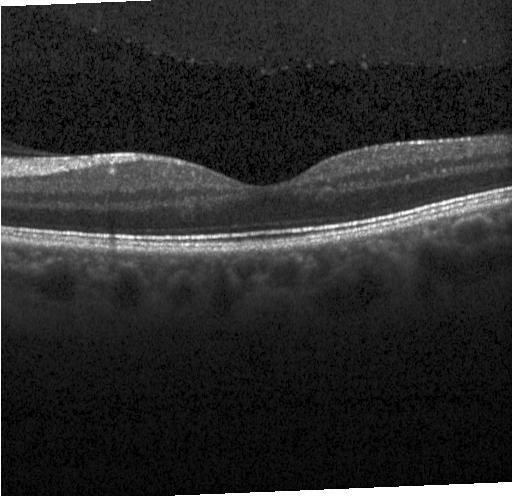

Optical coherence tomography scan
The scan shows no choroidal neovascularization, no diabetic macular edema, and no drusen.